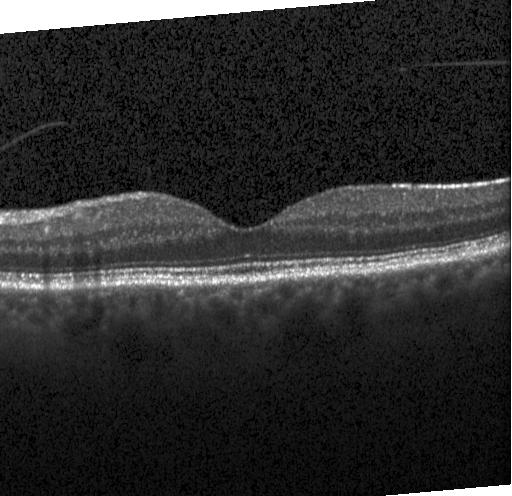 OCT finding: no choroidal neovascularization, no diabetic macular edema, and no drusen.